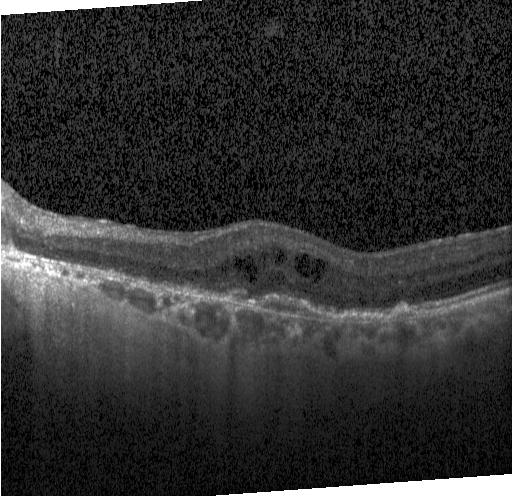 Optical coherence tomography scan; Heidelberg Spectralis; centered on the fovea. OCT finding: CNV.